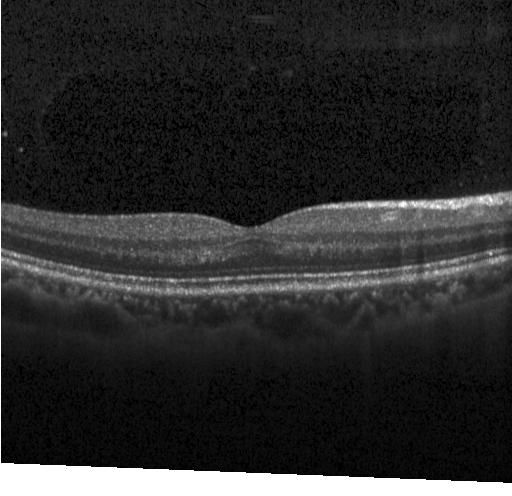

Heidelberg Spectralis OCT system · SD-OCT · retinal OCT B-scan
Finding: neither choroidal neovascularization, diabetic macular edema, nor drusen.